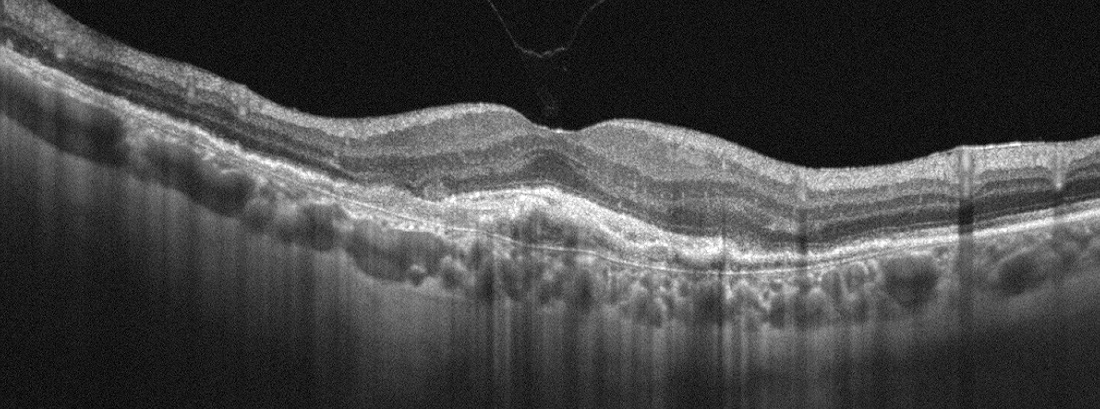

Macular OCT demonstrating age-related macular degeneration.